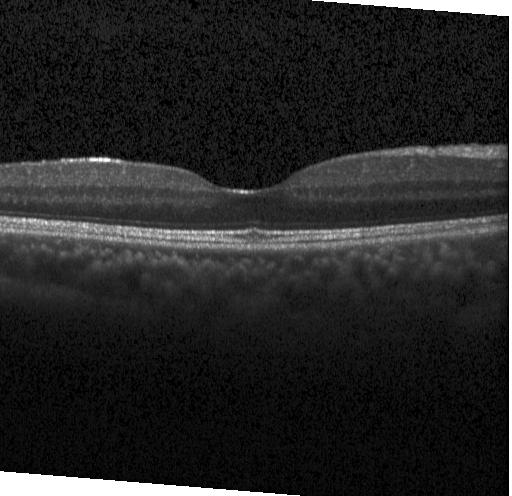
OCT B-scan — Finding: no CNV, no DME, and no drusen.